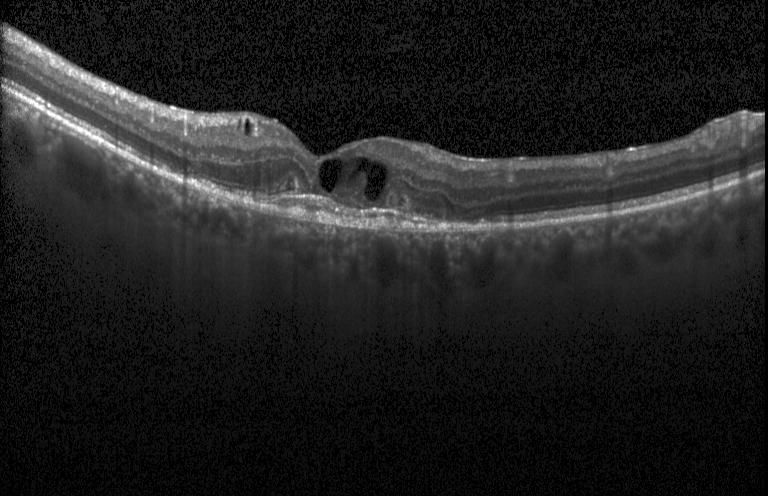
Diagnosis: CNV.